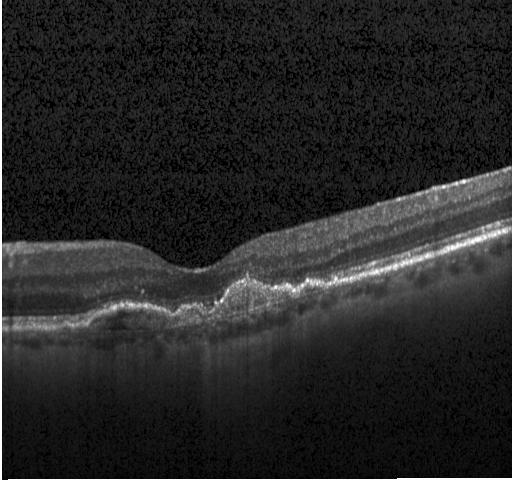
Spectral-domain optical coherence tomography · Heidelberg Spectralis OCT system · optical coherence tomography B-scan. Impression: a choroidal neovascular membrane.